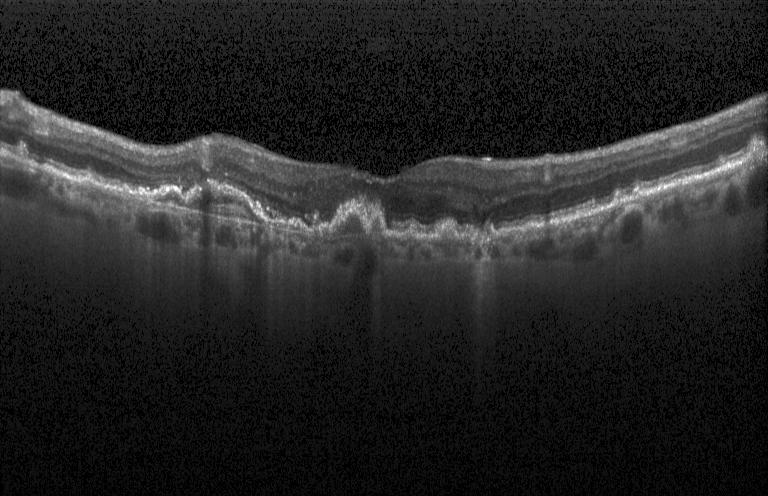

Retinal OCT cross-section
Drusen.